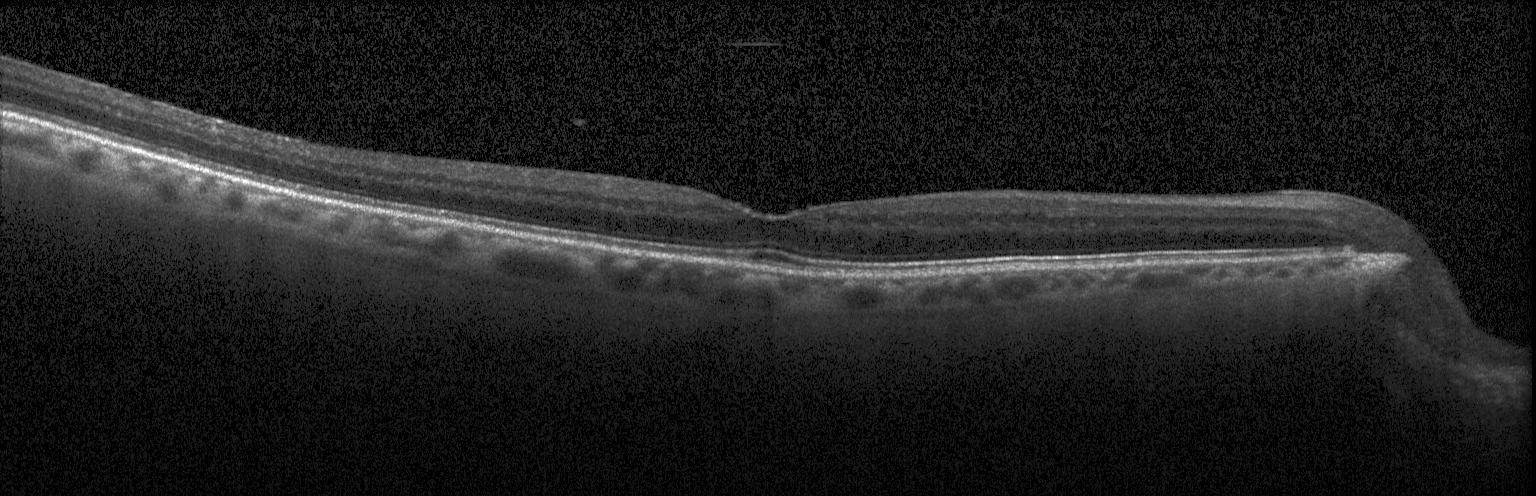 Macular OCT demonstrating no CNV, DME, or drusen.